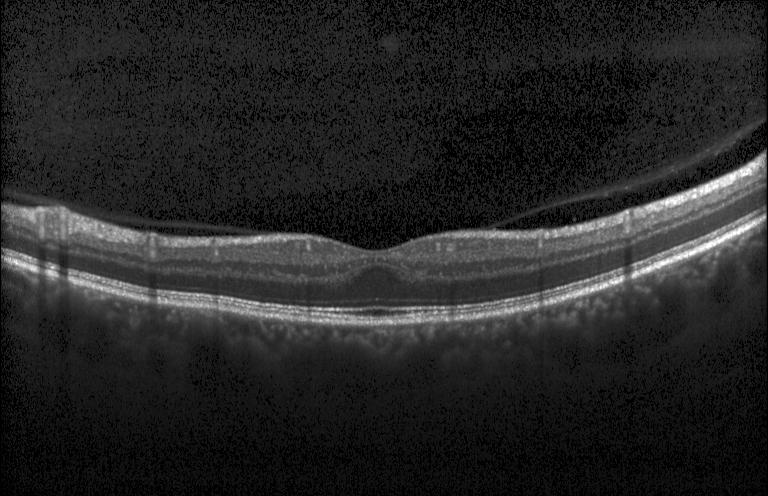

Assessment: no CNV, DME, or drusen.